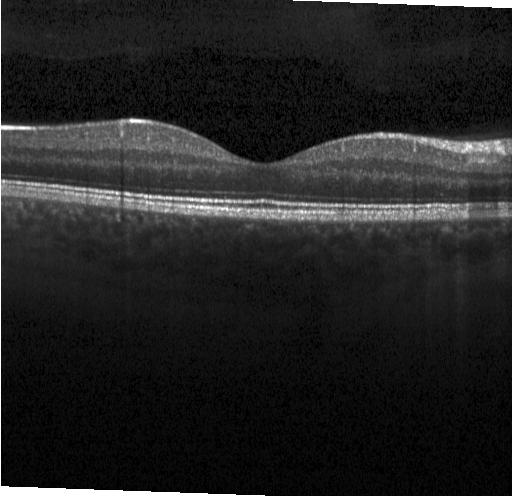
Fovea-centered. SD-OCT. OCT B-scan.
Impression: neither choroidal neovascularization, diabetic macular edema, nor drusen.